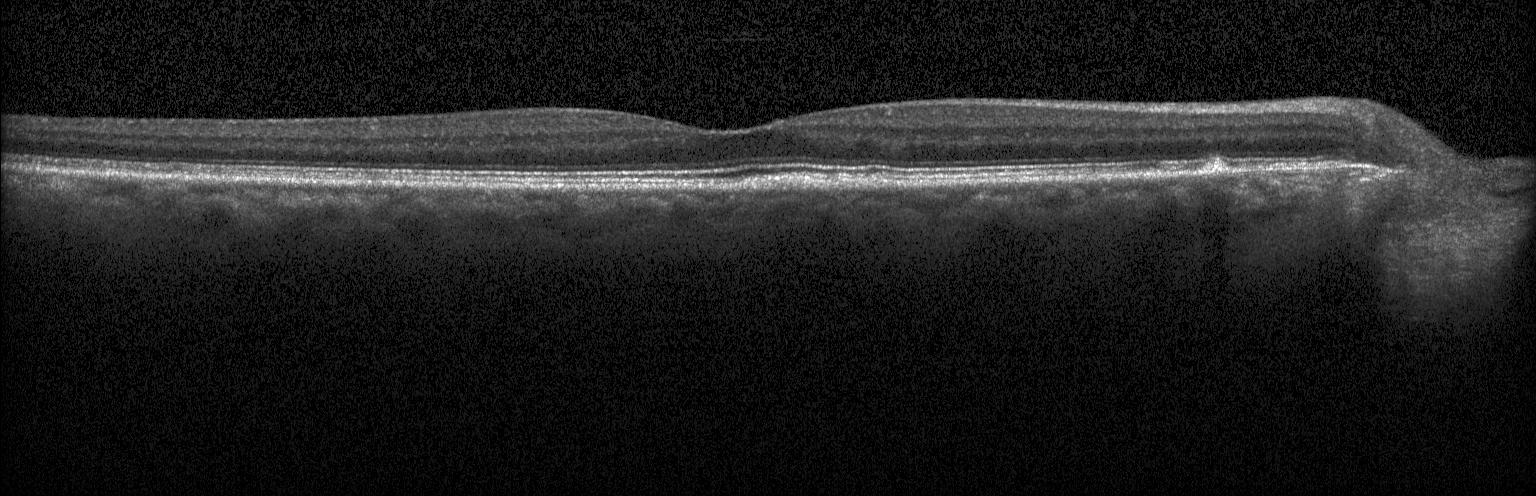 Impression: sub-RPE drusenoid deposits.